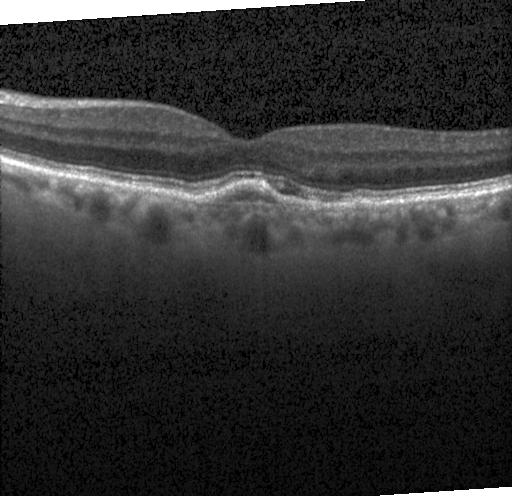
Optical coherence tomography scan. The scan shows choroidal neovascularization.